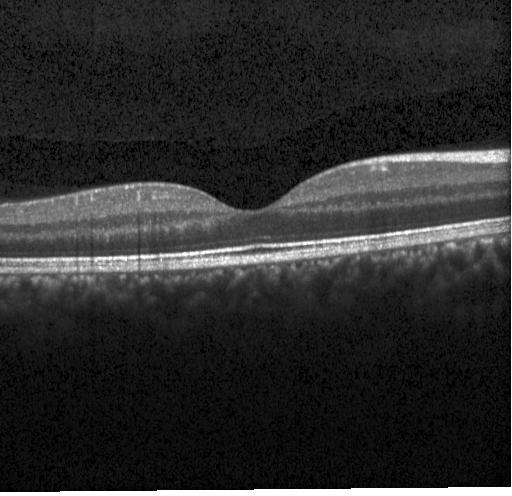

Through the macula, optical coherence tomography B-scan — The scan shows no choroidal neovascularization, no diabetic macular edema, and no drusen.